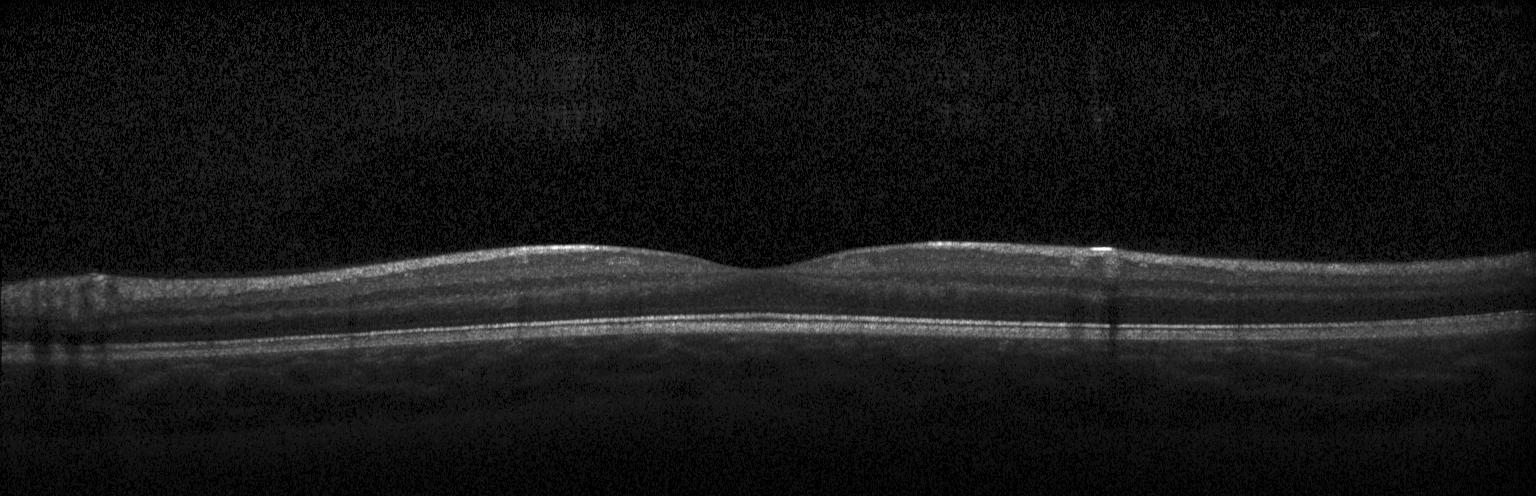

OCT B-scan, macular scan, spectral-domain optical coherence tomography, instrument: Heidelberg Spectralis.
Macular OCT: no evidence of choroidal neovascularization, diabetic macular edema, or drusen.